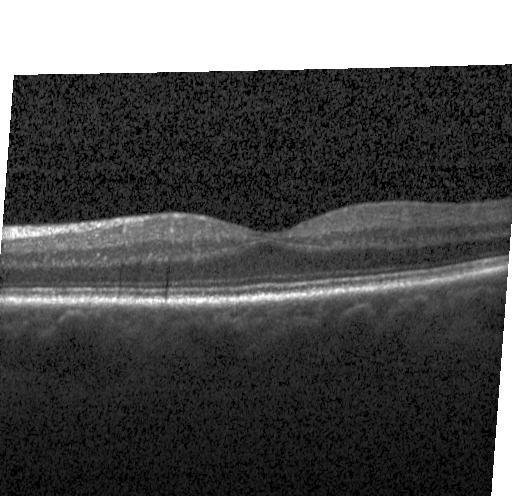

Retinal OCT cross-section.
Diagnosis: no choroidal neovascularization, no diabetic macular edema, and no drusen.